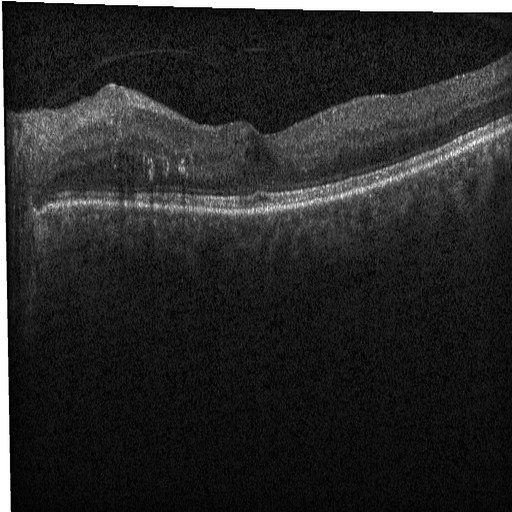 OCT line scan · horizontal scan through the fovea · spectral-domain optical coherence tomography.
Impression: diabetic macular edema (DME).